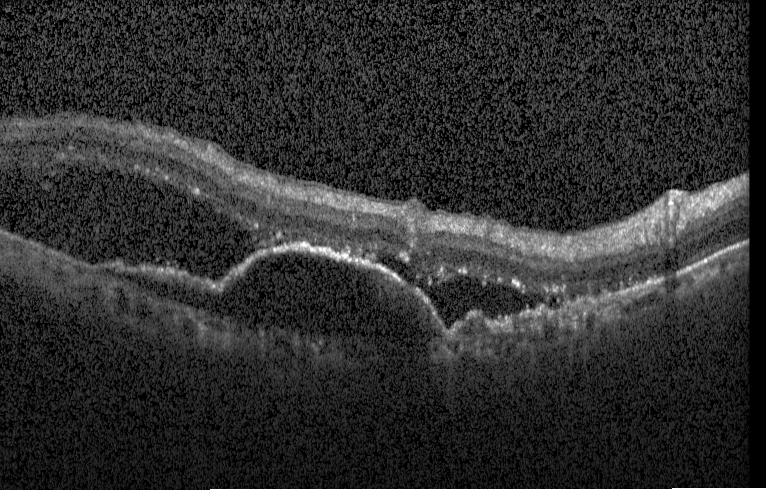
Spectral-domain optical coherence tomography. OCT line scan.
This B-scan demonstrates CNV.